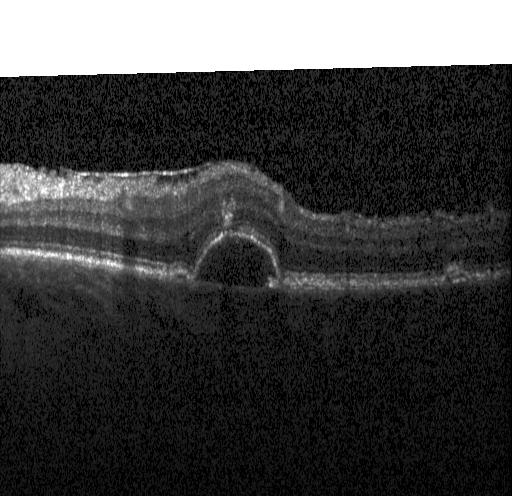 Instrument: Heidelberg Spectralis · horizontal scan through the fovea · retinal OCT B-scan · spectral-domain optical coherence tomography — The scan shows choroidal neovascularization.